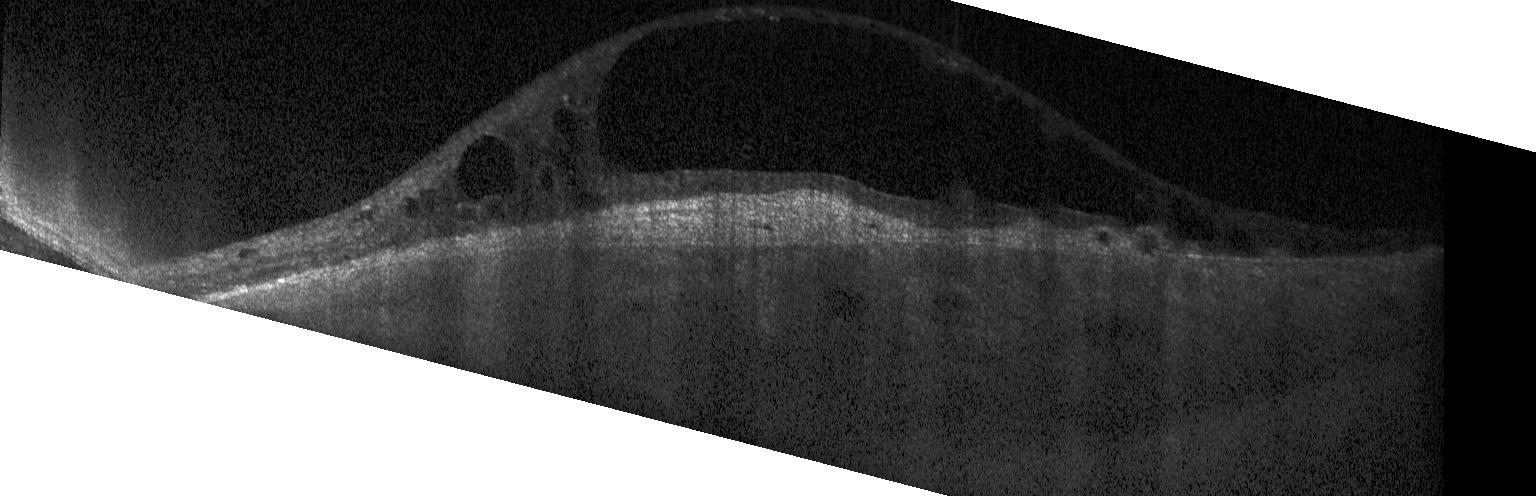 Diagnosis: choroidal neovascularization.